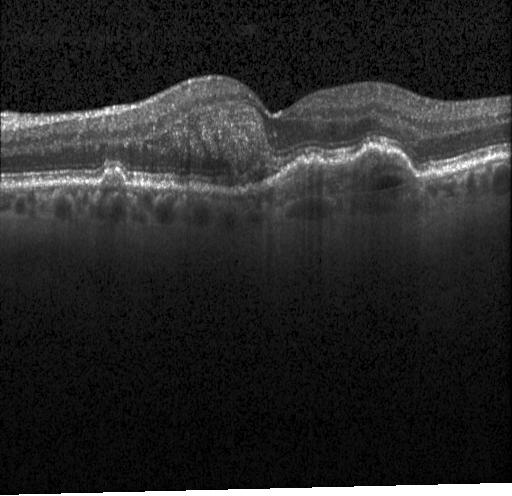
Choroidal neovascularization.